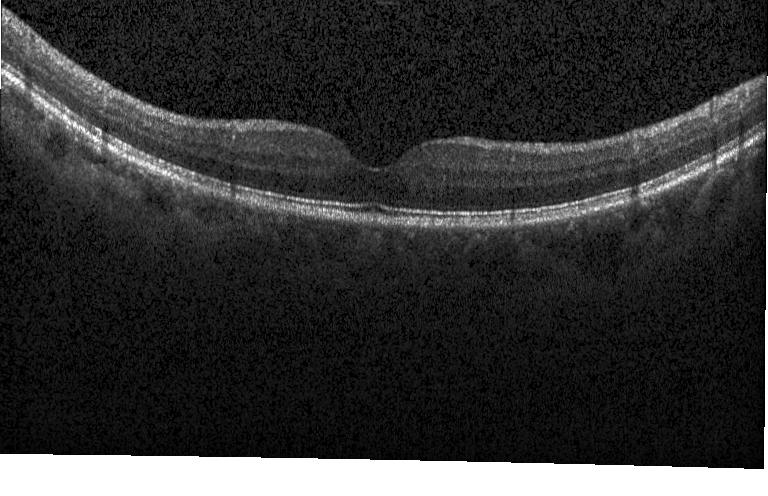

The scan shows no evidence of choroidal neovascularization, diabetic macular edema, or drusen.